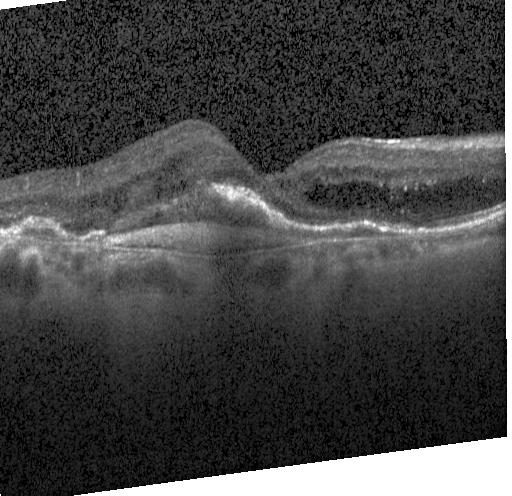 Impression: a choroidal neovascular membrane.